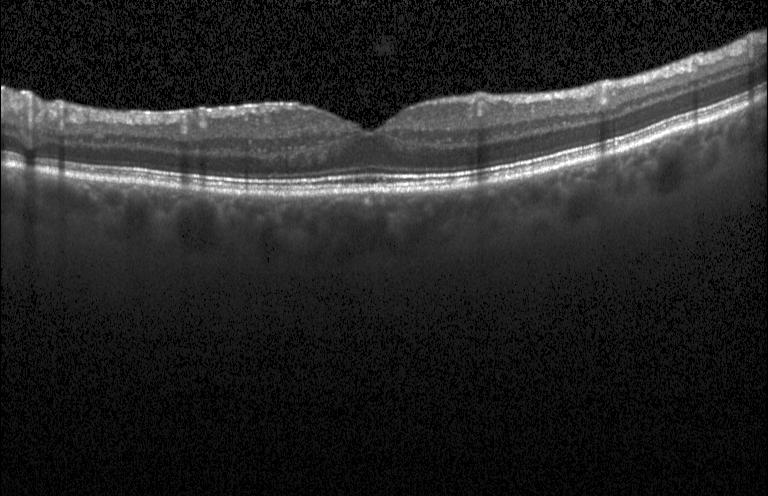
Impression: no evidence of choroidal neovascularization, diabetic macular edema, or drusen.